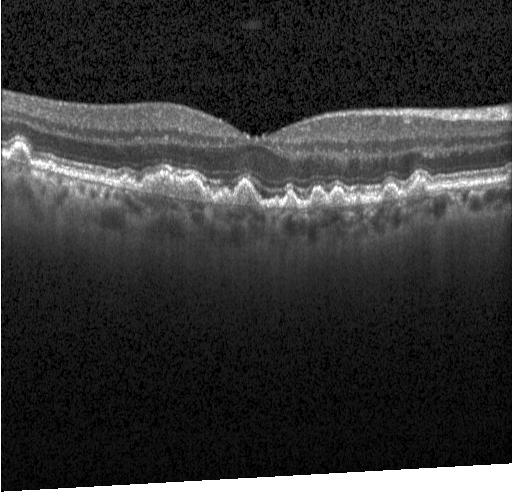 The scan shows sub-RPE drusenoid deposits.